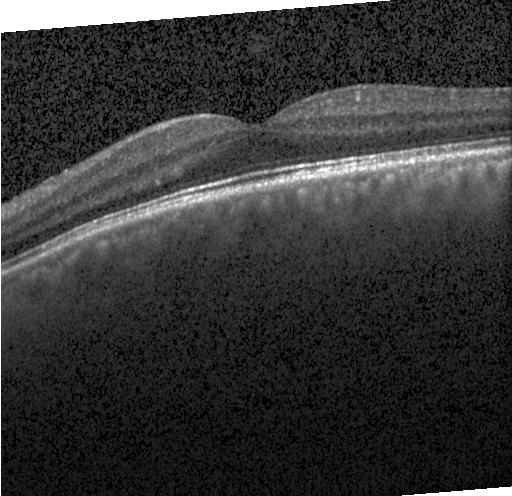

Macular scan · optical coherence tomography scan · Heidelberg Spectralis OCT system · spectral-domain OCT — The scan shows no choroidal neovascularization, diabetic macular edema, or drusen.